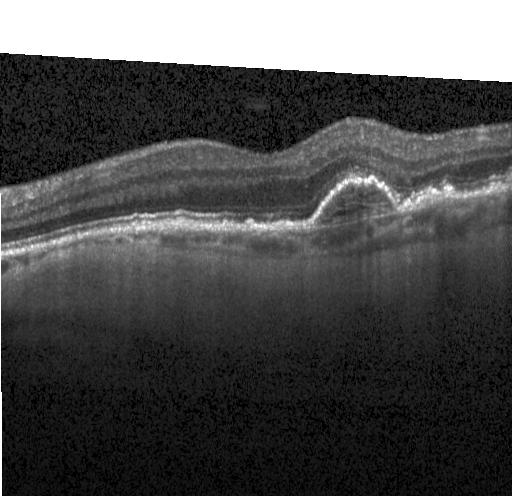

Retinal OCT cross-section, centered on the fovea, SD-OCT, instrument: Heidelberg Spectralis
Macular OCT: CNV.